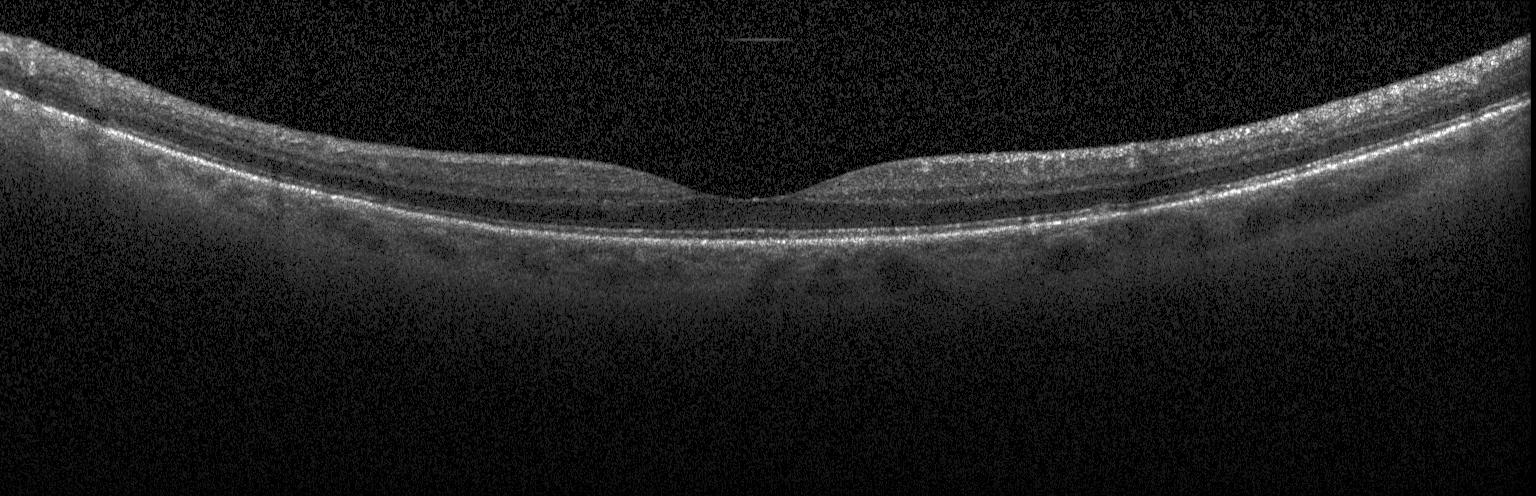 Diagnosis: no choroidal neovascularization, diabetic macular edema, or drusen.